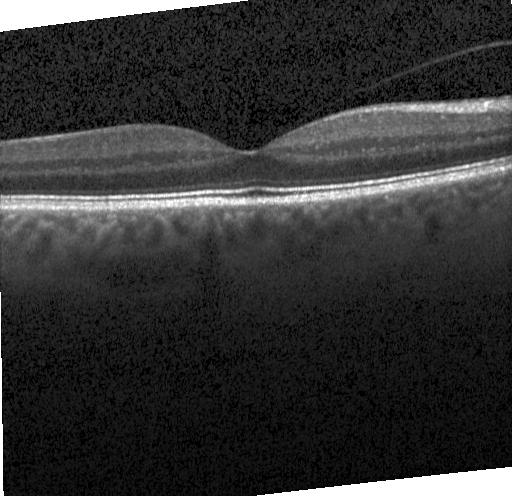

Spectral-domain OCT; horizontal scan through the fovea; optical coherence tomography scan; Heidelberg Spectralis. This B-scan demonstrates neither choroidal neovascularization, diabetic macular edema, nor drusen.